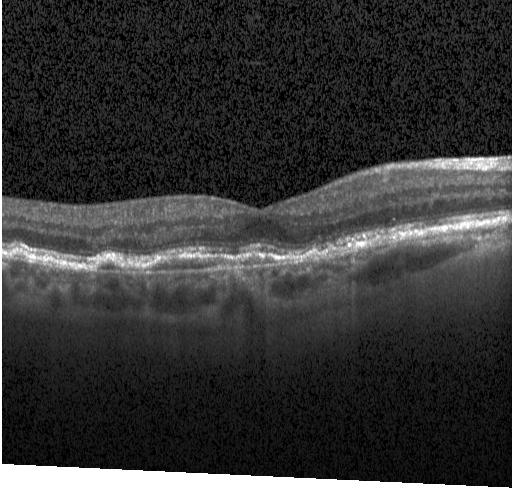
CNV.